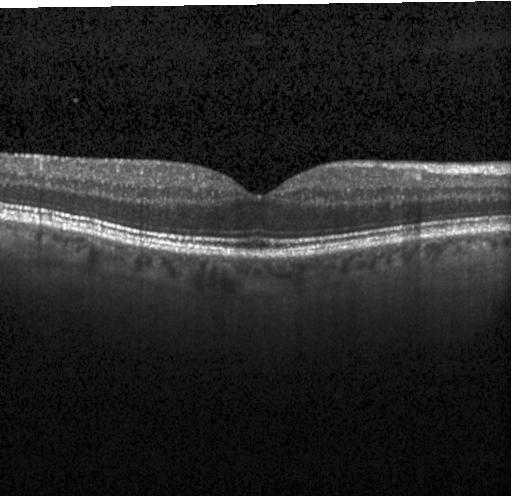
Retinal OCT cross-section showing no CNV, no DME, and no drusen.